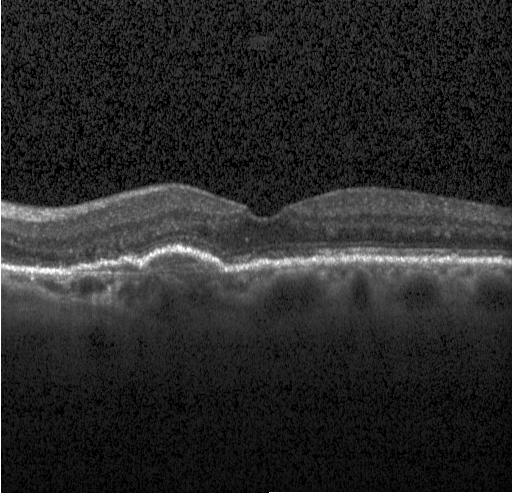 Retinal OCT cross-section showing a choroidal neovascular membrane.